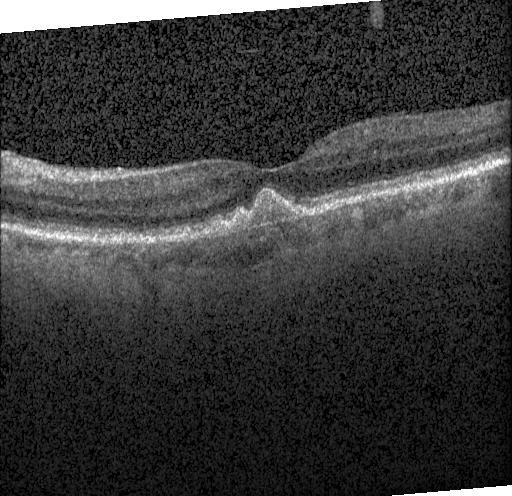
Finding: drusen.